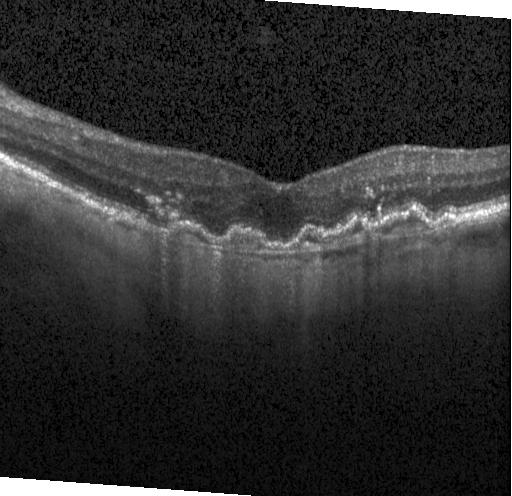
Optical coherence tomography B-scan; Heidelberg Spectralis. Assessment: choroidal neovascularization (CNV).